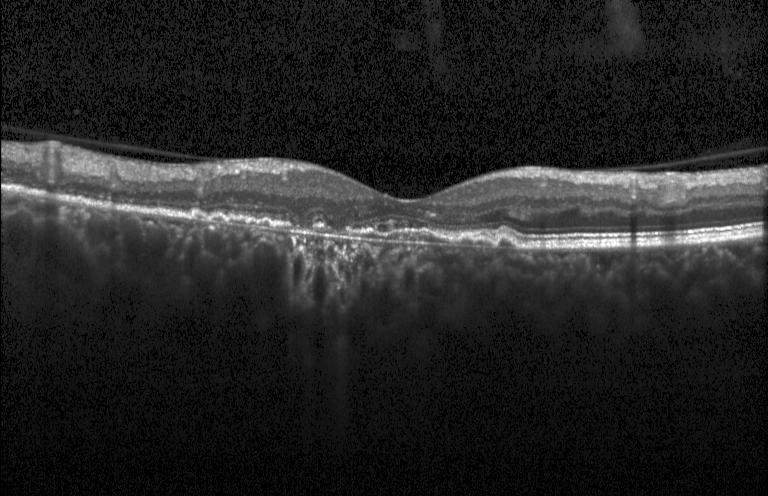

Optical coherence tomography scan. Heidelberg Spectralis. Centered on the fovea. SD-OCT — Finding: a choroidal neovascular membrane.